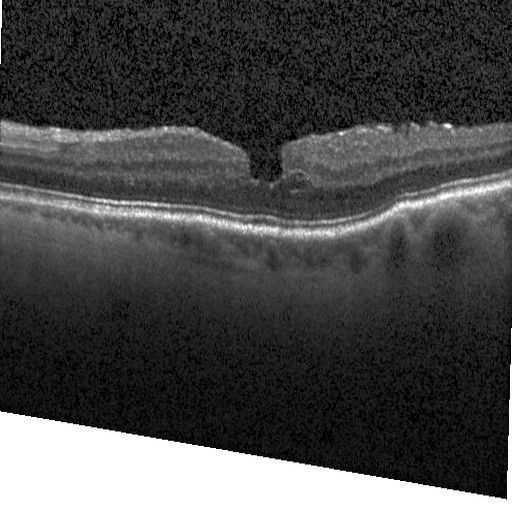 Spectral-domain OCT B-scan: DME.